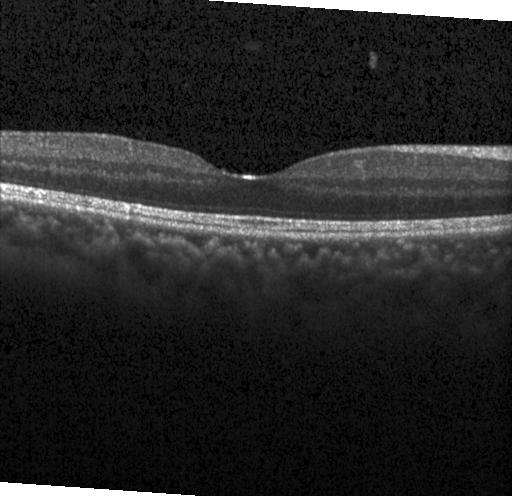 Spectral-domain optical coherence tomography. OCT B-scan. Fovea-centered. Diagnosis: no evidence of choroidal neovascularization, diabetic macular edema, or drusen.